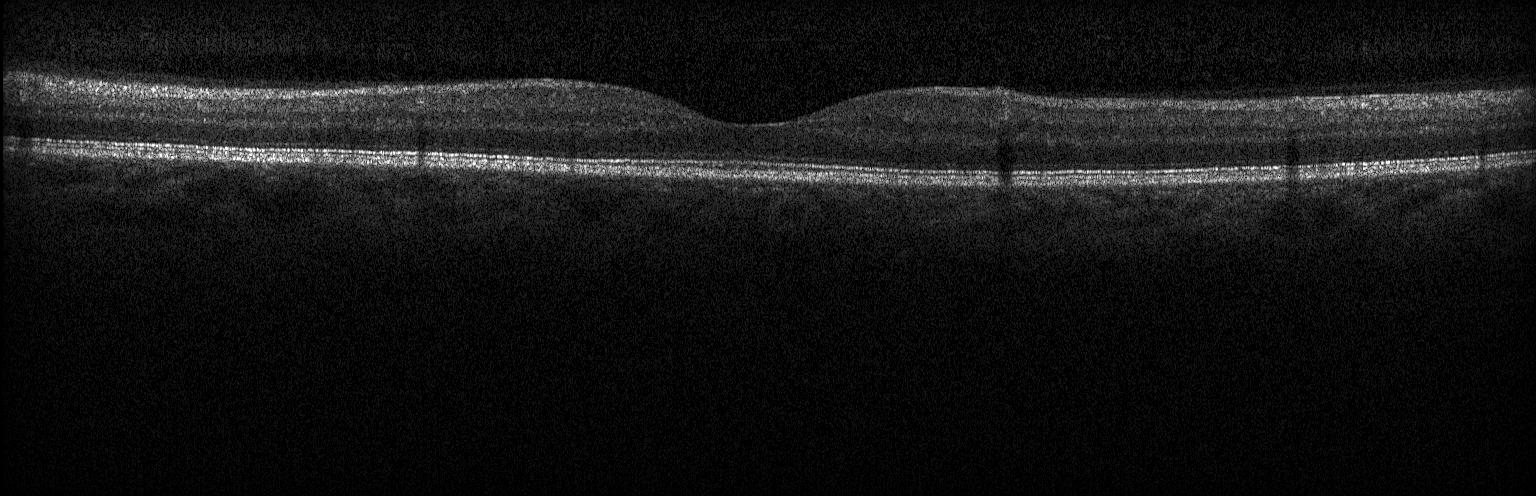
Acquired on a Heidelberg Spectralis, retinal OCT B-scan. Diagnosis: no choroidal neovascularization, no diabetic macular edema, and no drusen.